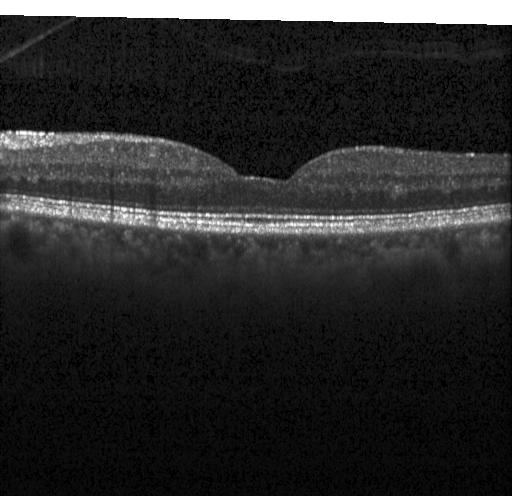

Fovea-centered · spectral-domain OCT · Heidelberg Spectralis · retinal OCT B-scan. Macular OCT: neither choroidal neovascularization, diabetic macular edema, nor drusen.